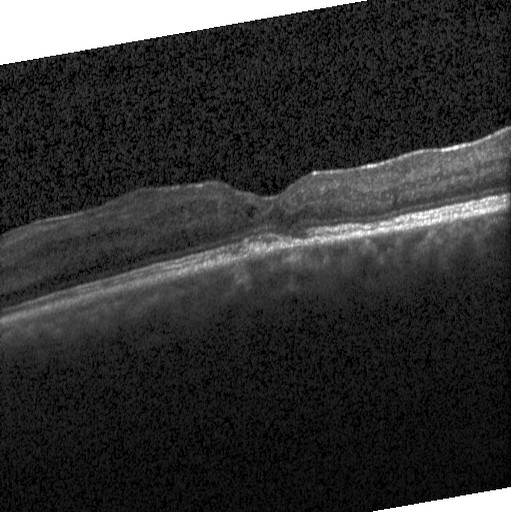 Diagnosis: diabetic macular edema.